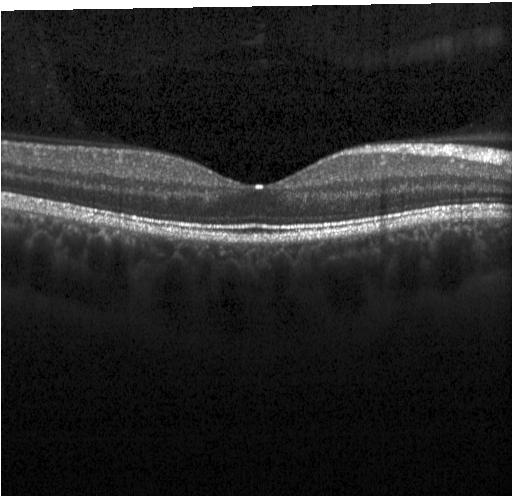

Heidelberg Spectralis, centered on the fovea, OCT line scan.
Impression: no choroidal neovascularization, diabetic macular edema, or drusen.